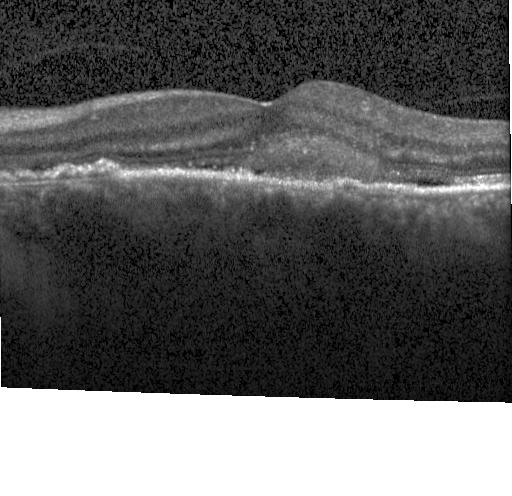

Spectral-domain OCT; optical coherence tomography scan; through the macula; Heidelberg Spectralis OCT system
Impression: CNV.